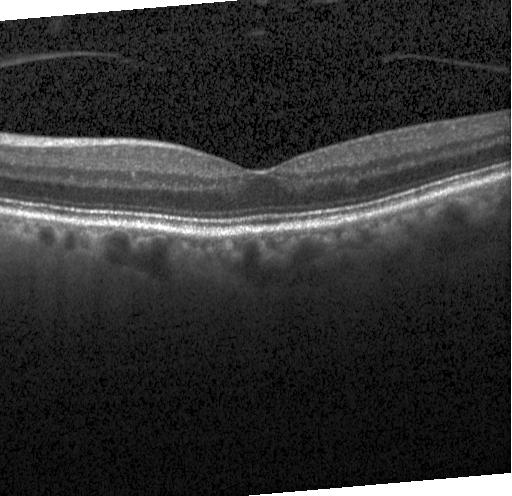 Instrument: Heidelberg Spectralis, horizontal scan through the fovea, OCT line scan — Impression: no choroidal neovascularization, no diabetic macular edema, and no drusen.